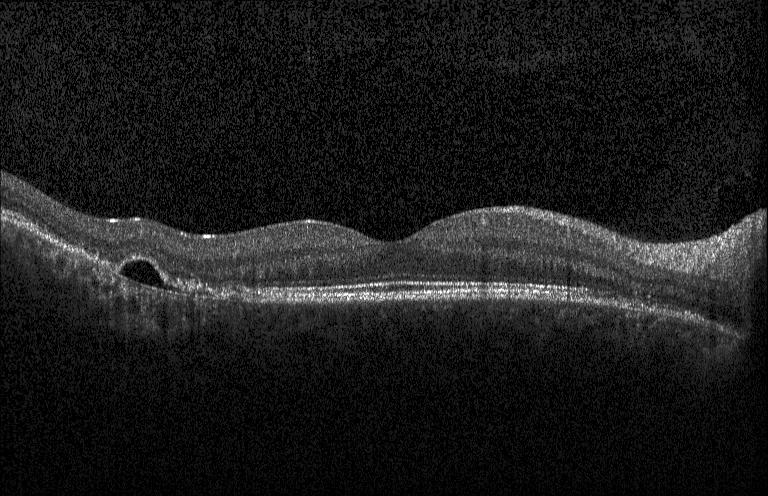

Retinal OCT B-scan. The scan shows a choroidal neovascular membrane.